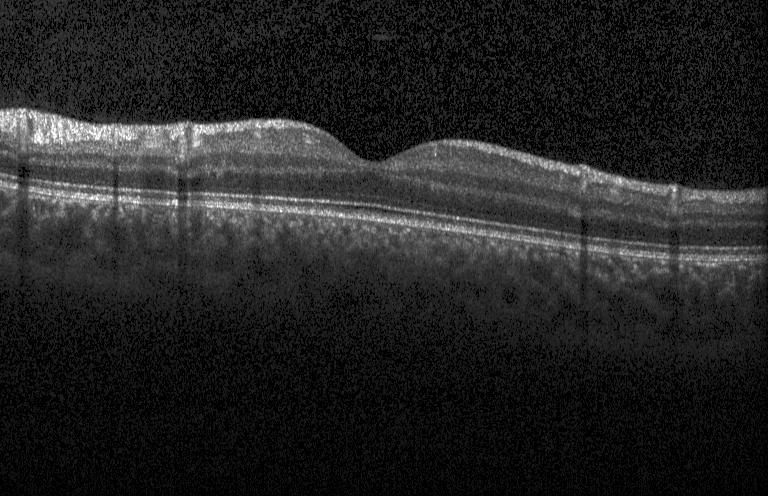

Spectral-domain OCT B-scan: no choroidal neovascularization, no diabetic macular edema, and no drusen.